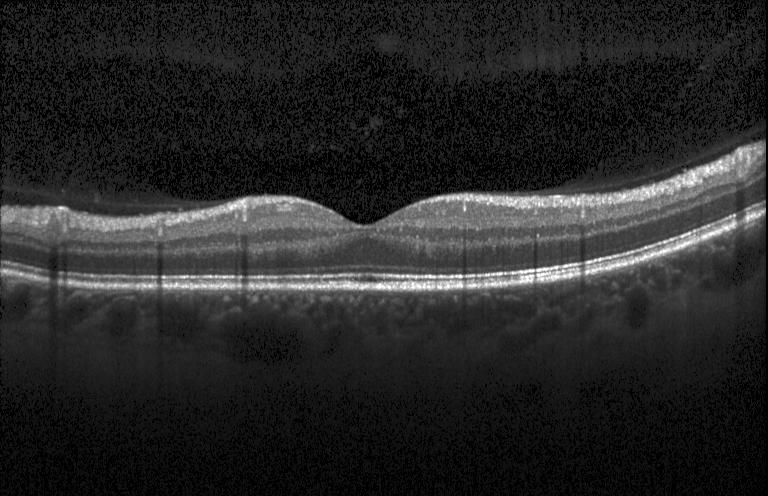

OCT finding: neither choroidal neovascularization, diabetic macular edema, nor drusen.